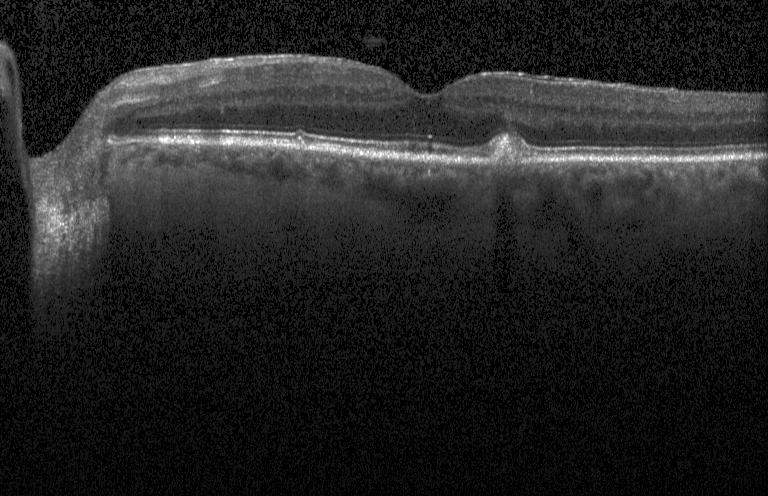 Instrument: Heidelberg Spectralis · OCT line scan · spectral-domain OCT
Diagnosis: sub-RPE drusenoid deposits.